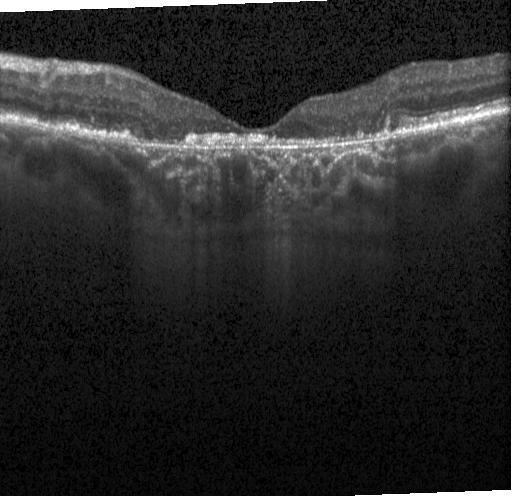
Finding: a choroidal neovascular membrane.